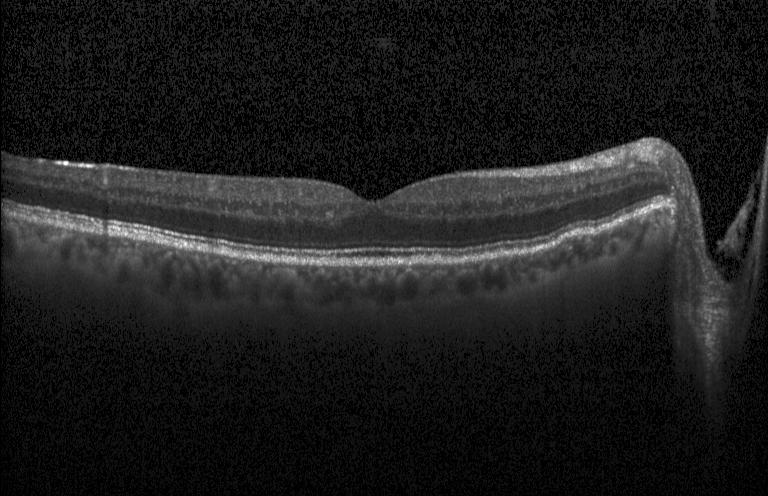
Retinal OCT cross-section, centered on the fovea, SD-OCT — Impression: no evidence of choroidal neovascularization, diabetic macular edema, or drusen.